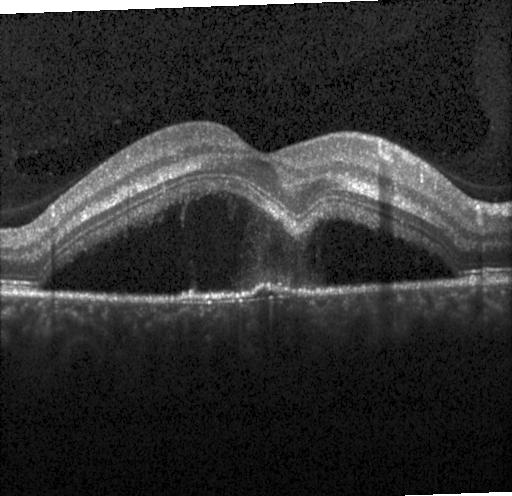

SD-OCT, through the macula, instrument: Heidelberg Spectralis, retinal OCT cross-section. Diagnosis: CNV.